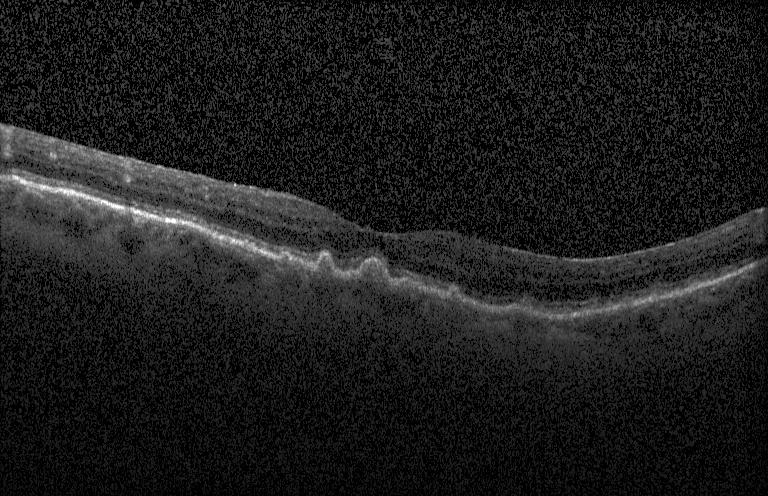
Optical coherence tomography B-scan — Assessment: sub-RPE drusenoid deposits.